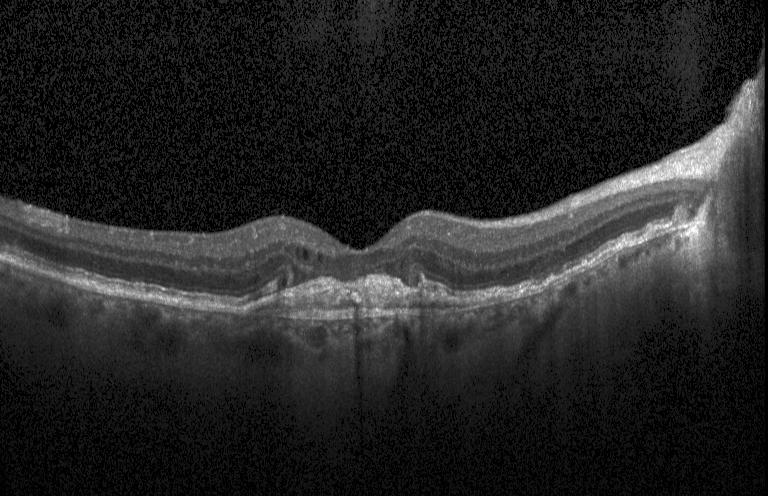

OCT line scan. Spectral-domain optical coherence tomography — Finding: a choroidal neovascular membrane.